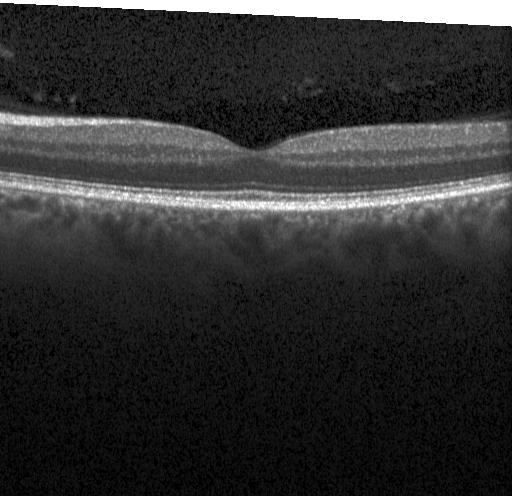 Retinal OCT B-scan — The scan shows no choroidal neovascularization, no diabetic macular edema, and no drusen.